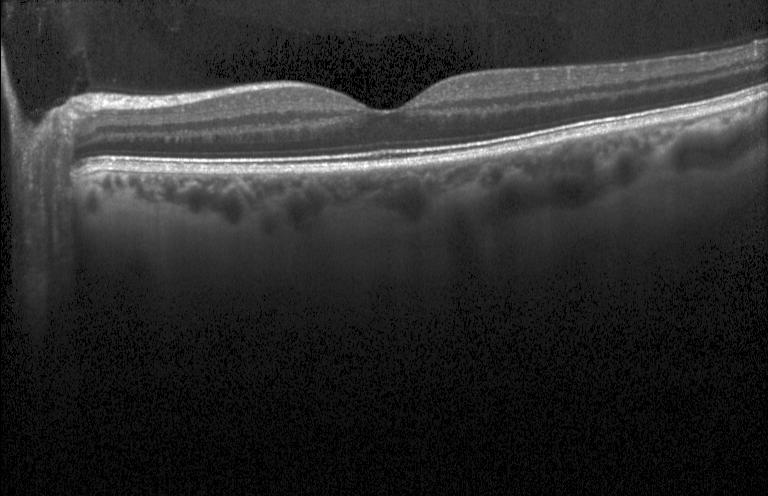 OCT B-scan. Centered on the fovea — Diagnosis: no evidence of choroidal neovascularization, diabetic macular edema, or drusen.